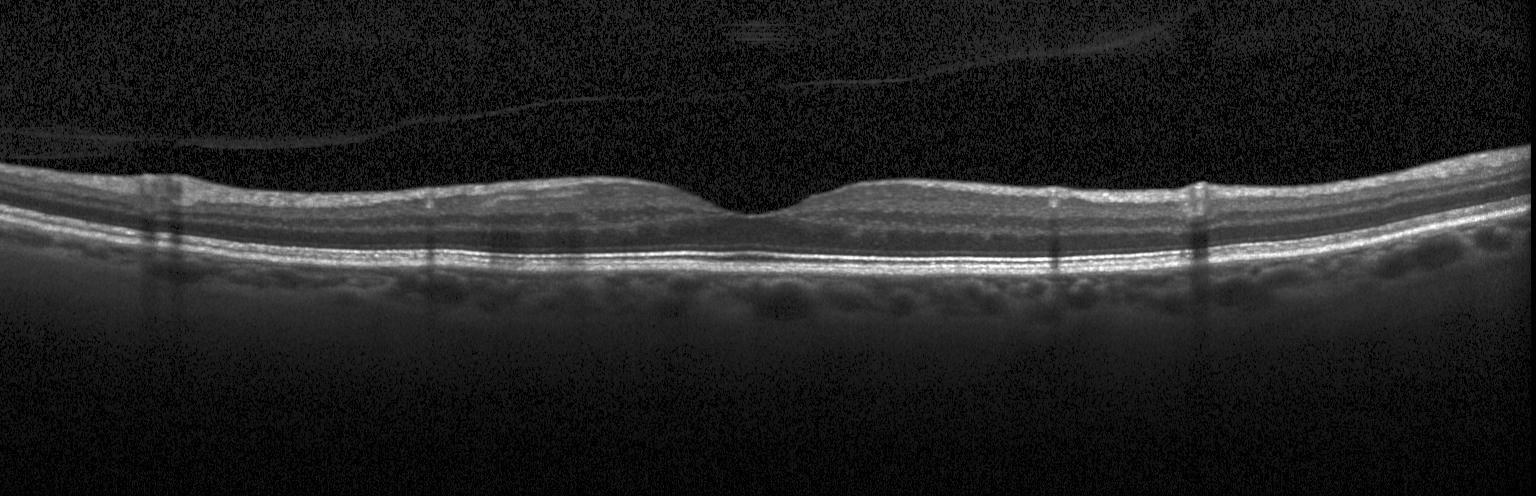 OCT line scan.
Finding: no CNV, DME, or drusen.